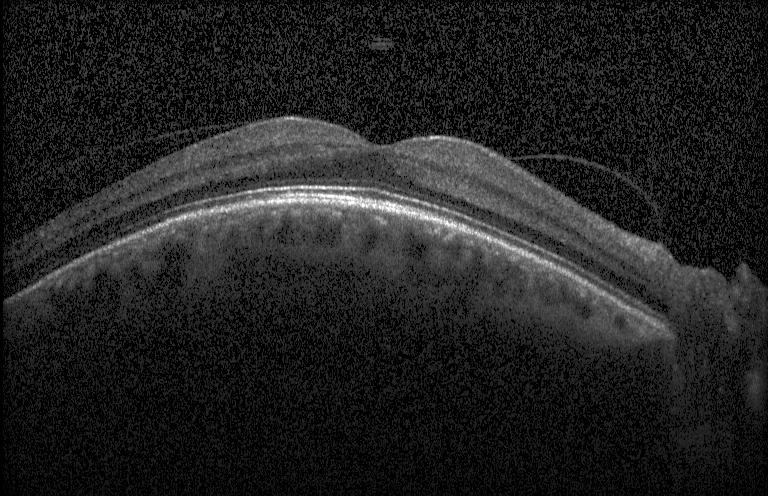

Retinal OCT cross-section.
Macular OCT: no CNV, DME, or drusen.